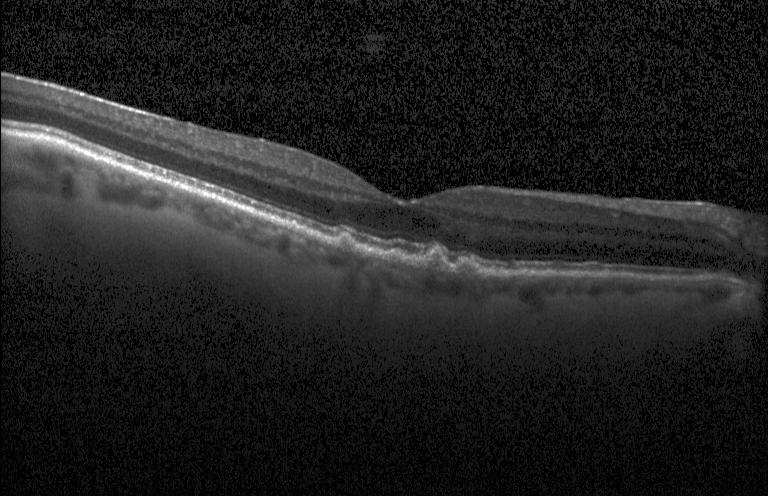
Acquired on a Heidelberg Spectralis, centered on the fovea, SD-OCT, OCT B-scan.
Dx: sub-RPE drusenoid deposits.